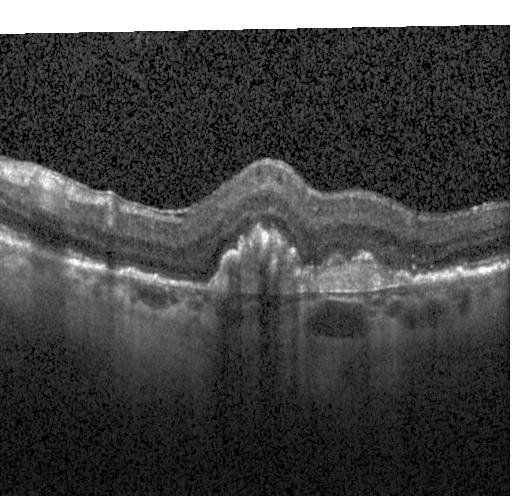 Dx: choroidal neovascularization.